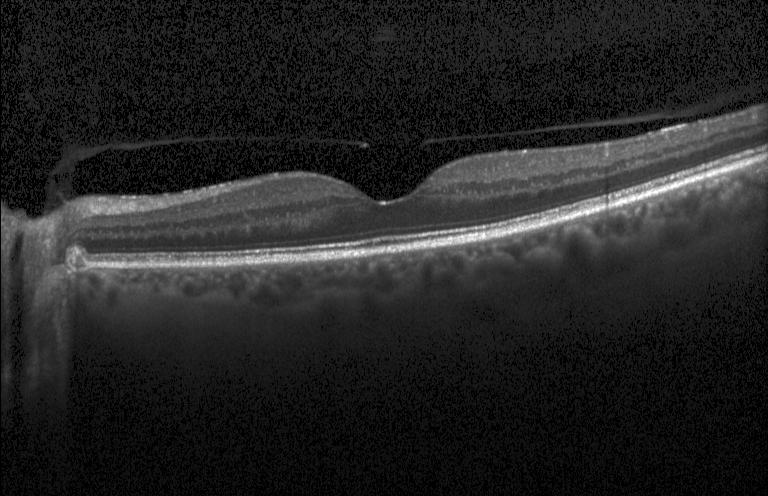
Retinal OCT B-scan · spectral-domain OCT · fovea-centered. Assessment: no choroidal neovascularization, diabetic macular edema, or drusen.